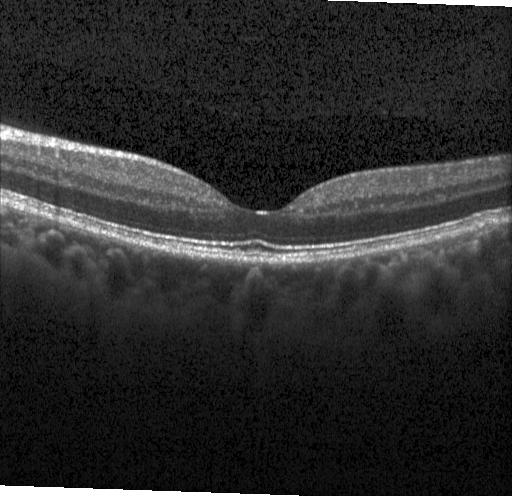
OCT B-scan; horizontal scan through the fovea; spectral-domain OCT
Finding: no CNV, no DME, and no drusen.